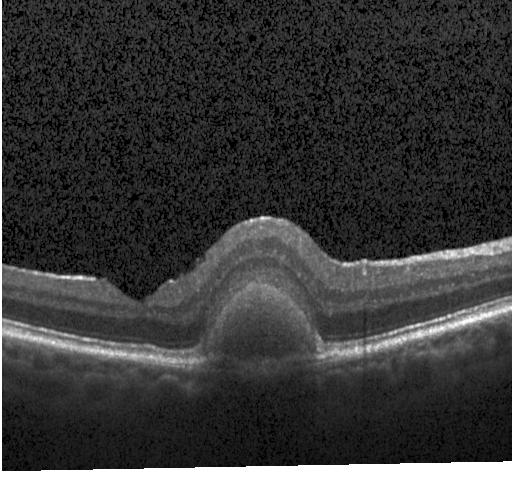 Spectral-domain OCT, OCT line scan. Choroidal neovascularization.